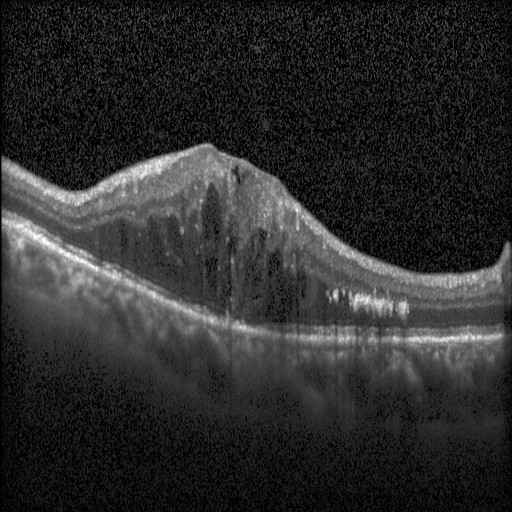
Dx: DME.